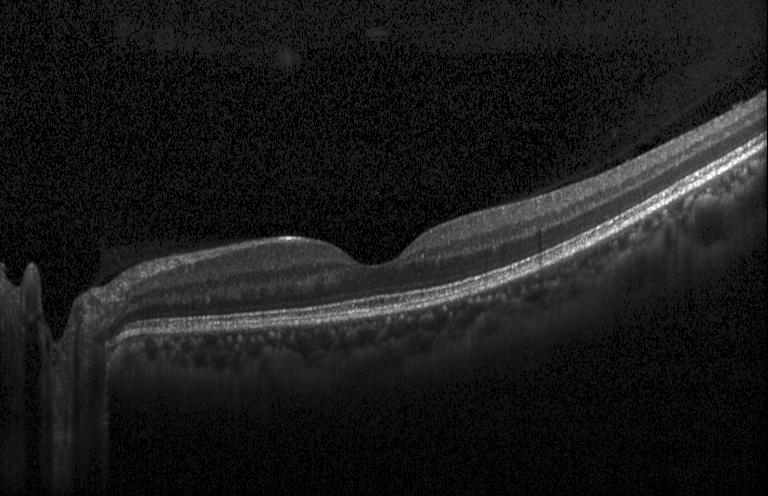
Spectral-domain OCT B-scan: no choroidal neovascularization, diabetic macular edema, or drusen.